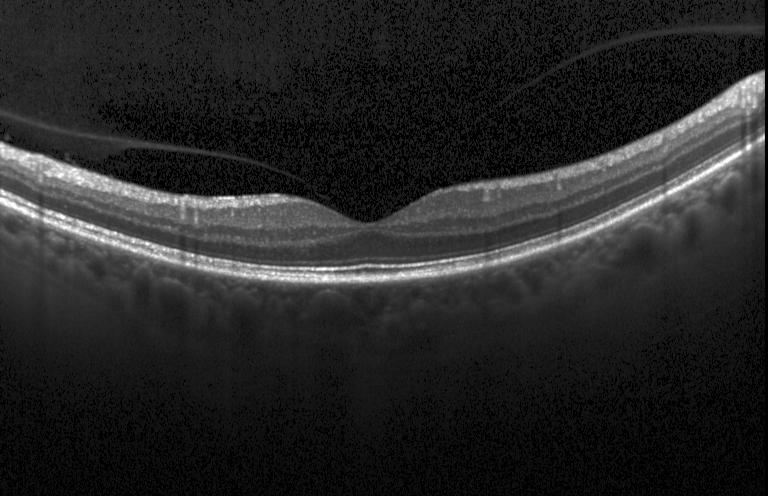 Retinal OCT cross-section. Impression: no choroidal neovascularization, diabetic macular edema, or drusen.